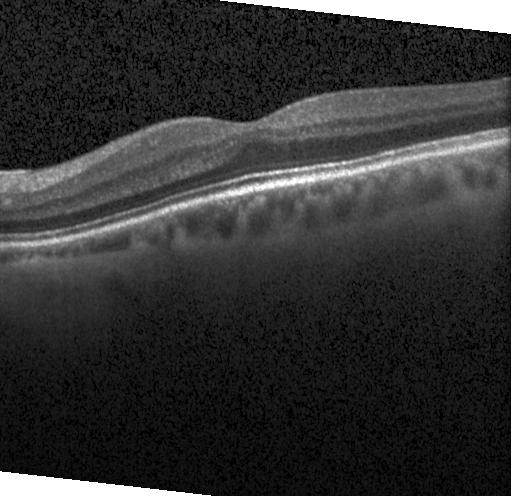
Diagnosis: no CNV, DME, or drusen.